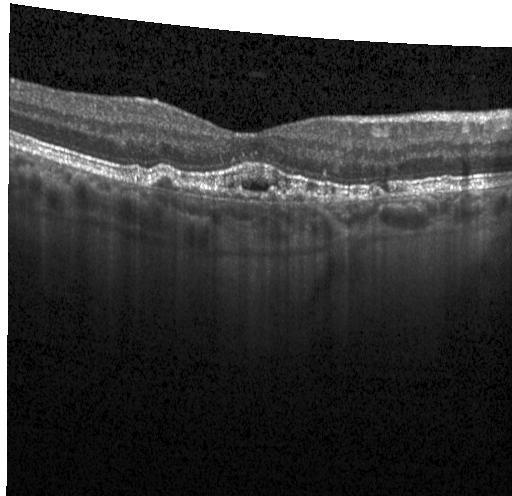
Spectral-domain optical coherence tomography, retinal OCT B-scan, centered on the fovea.
Assessment: choroidal neovascularization.